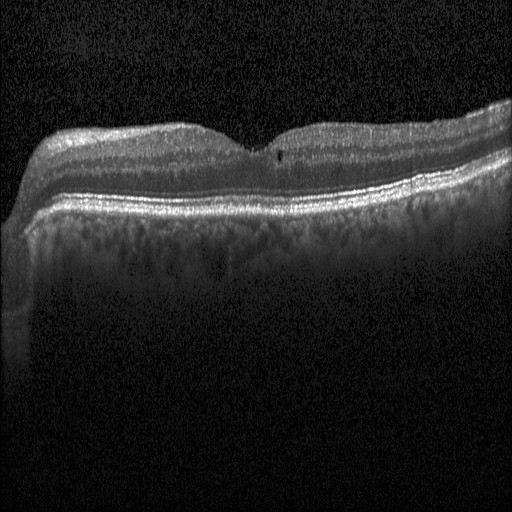

Retinal OCT cross-section.
Impression: diabetic macular edema (DME).